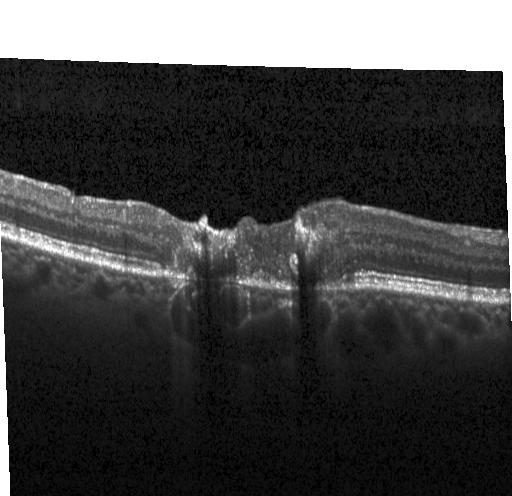
Macular OCT demonstrating CNV.